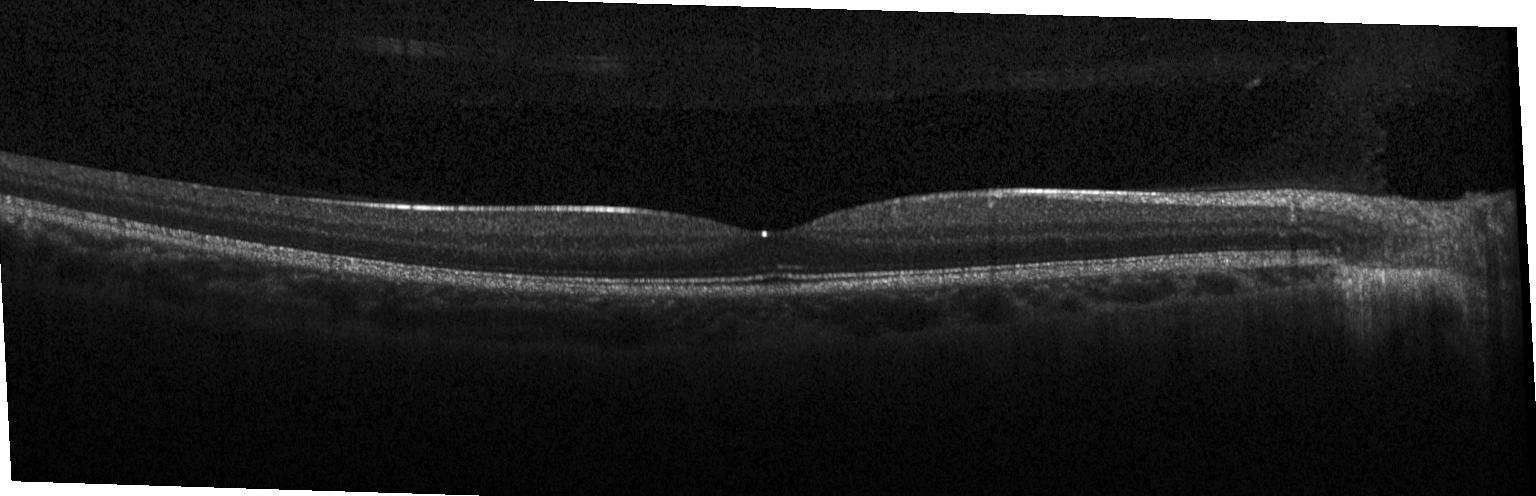
OCT B-scan; spectral-domain OCT; instrument: Heidelberg Spectralis; centered on the fovea
Diagnosis: neither choroidal neovascularization, diabetic macular edema, nor drusen.